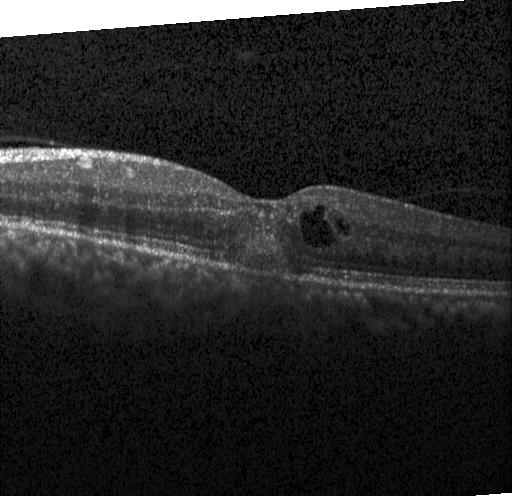 Horizontal scan through the fovea · SD-OCT · OCT line scan · instrument: Heidelberg Spectralis — A choroidal neovascular membrane.